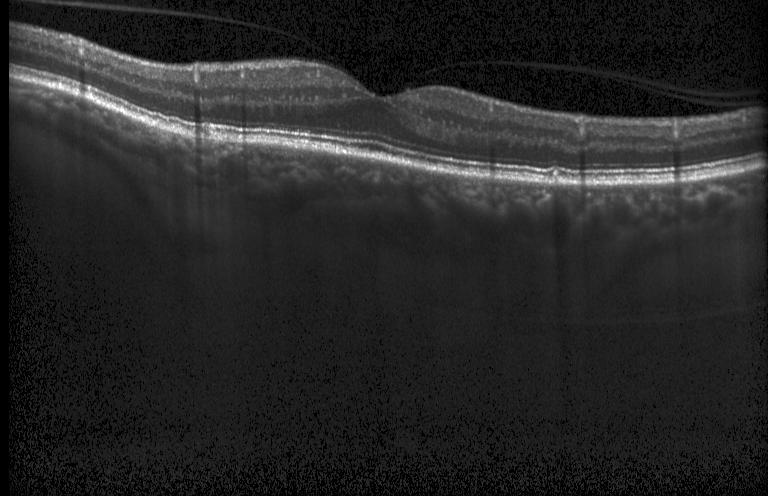

Retinal OCT B-scan — Assessment: no choroidal neovascularization, no diabetic macular edema, and no drusen.